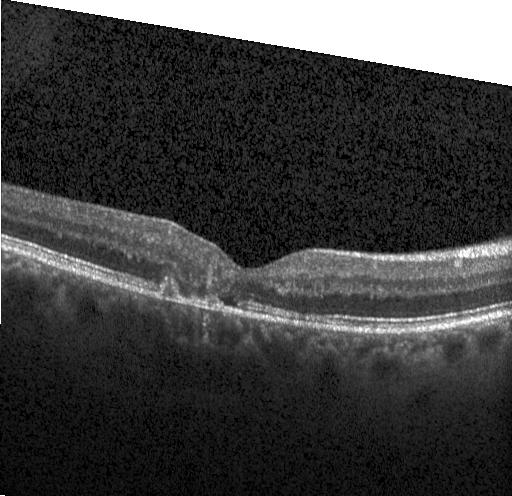

Macular scan. SD-OCT. Retinal OCT B-scan. Heidelberg Spectralis. Impression: a choroidal neovascular membrane.